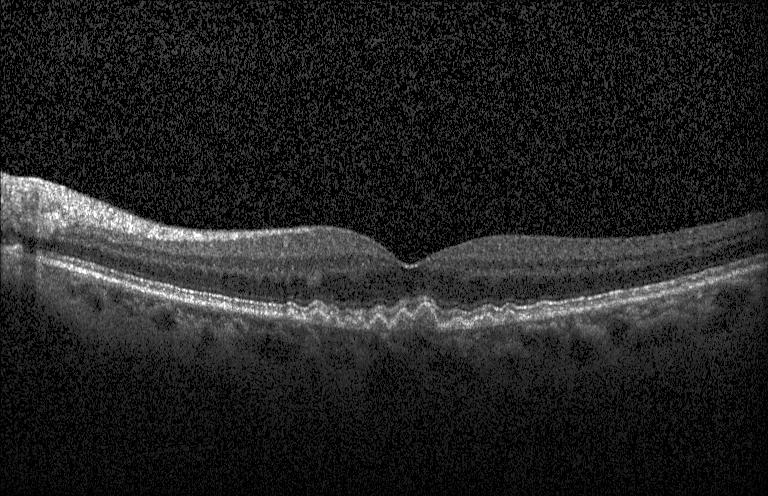

Drusen.